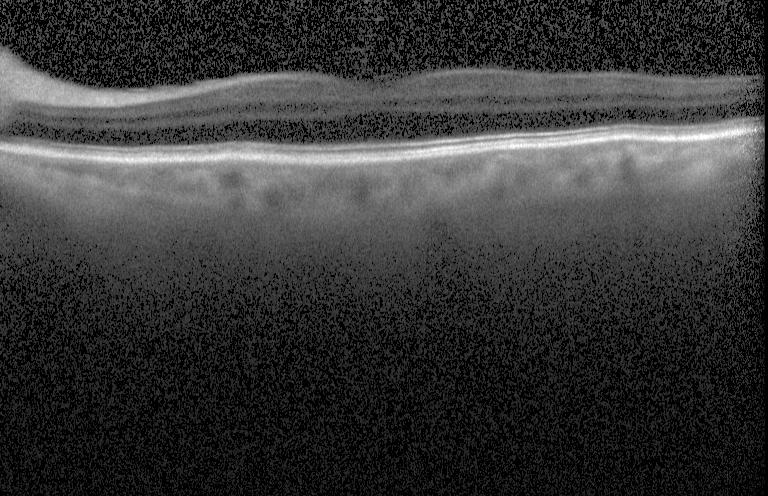 Instrument: Heidelberg Spectralis, retinal OCT cross-section.
Assessment: no choroidal neovascularization, diabetic macular edema, or drusen.